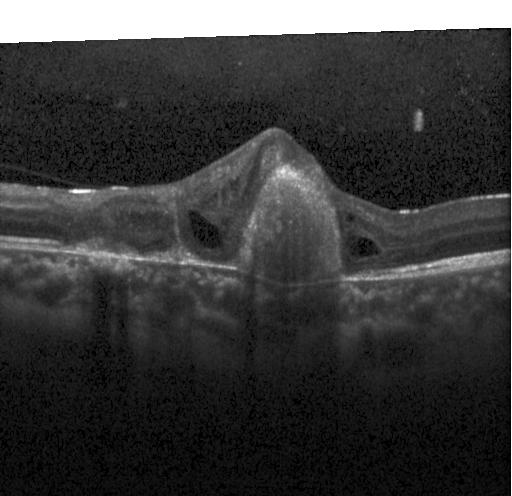 Optical coherence tomography scan — Impression: a choroidal neovascular membrane.